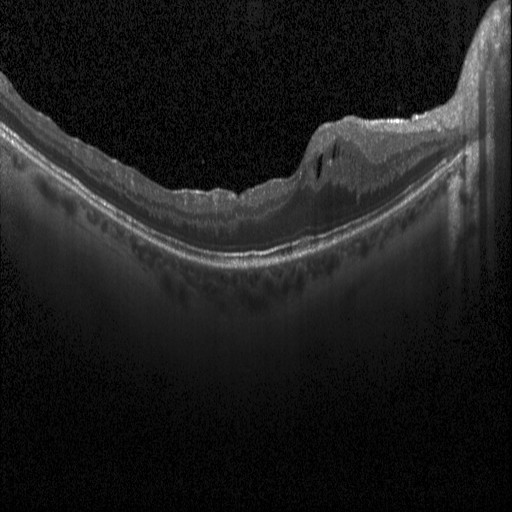

Heidelberg Spectralis OCT system; retinal OCT cross-section. Impression: diabetic macular edema (DME).